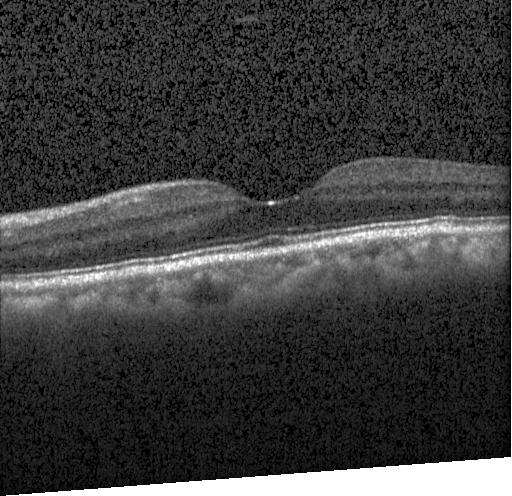

Macular scan · Heidelberg Spectralis · optical coherence tomography B-scan · spectral-domain optical coherence tomography. Diagnosis: no choroidal neovascularization, no diabetic macular edema, and no drusen.